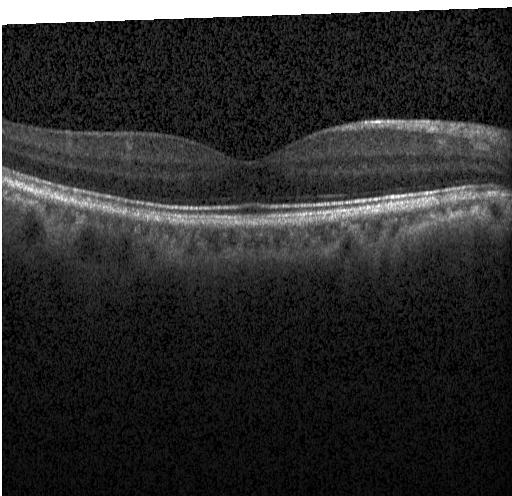
Finding: no choroidal neovascularization, no diabetic macular edema, and no drusen.